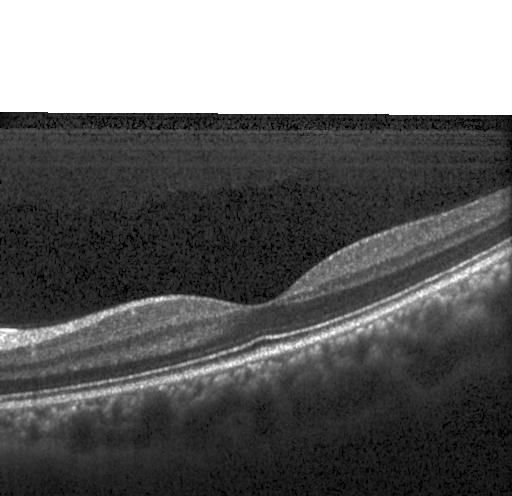

Impression: no evidence of choroidal neovascularization, diabetic macular edema, or drusen.